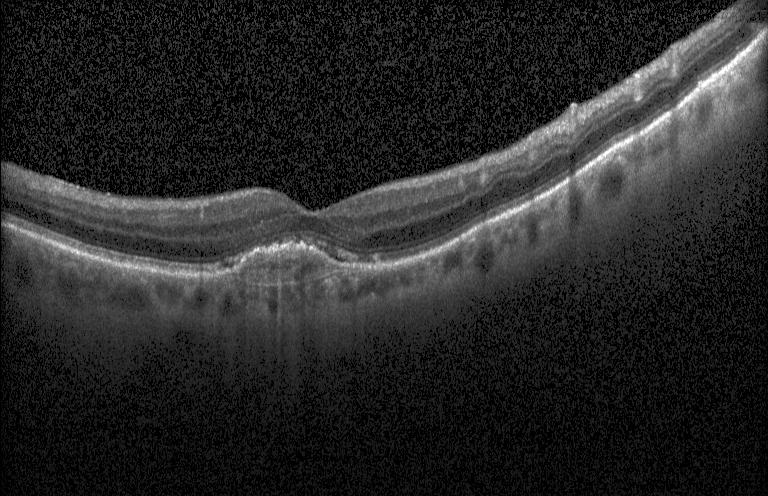 Retinal OCT B-scan · macular scan
Diagnosis: a choroidal neovascular membrane.